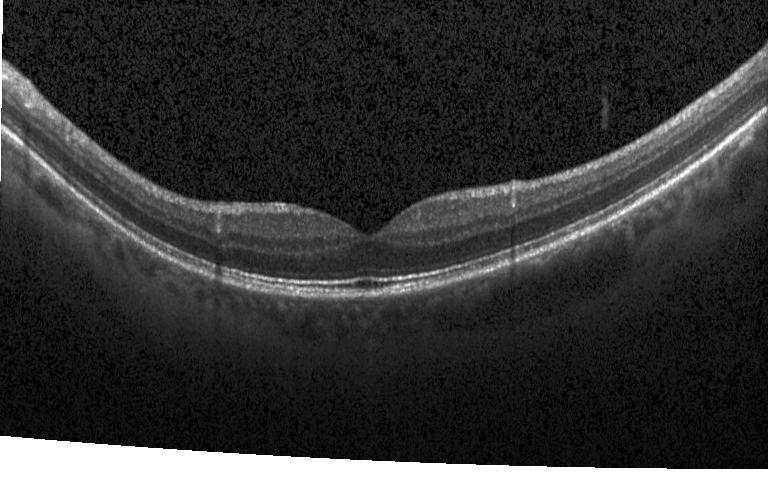 Spectral-domain OCT B-scan: no evidence of choroidal neovascularization, diabetic macular edema, or drusen.